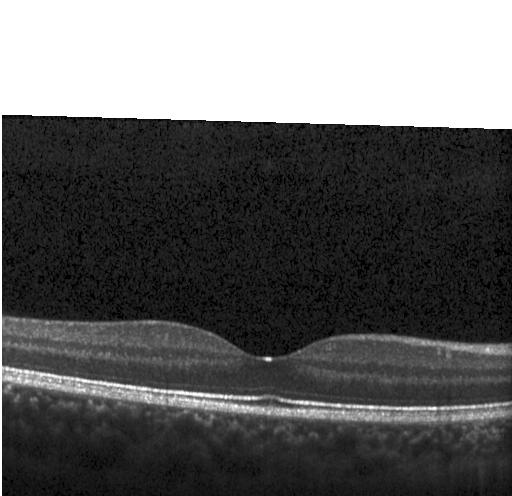
Fovea-centered, optical coherence tomography B-scan. The scan shows no choroidal neovascularization, diabetic macular edema, or drusen.